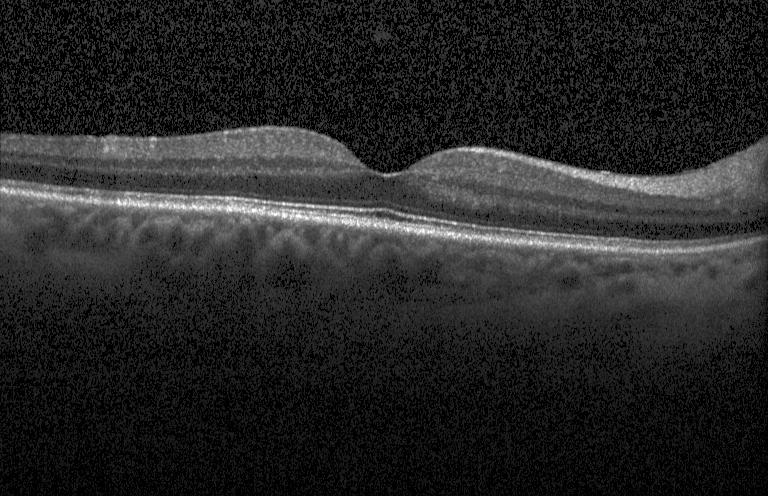 Macular OCT: no evidence of choroidal neovascularization, diabetic macular edema, or drusen.